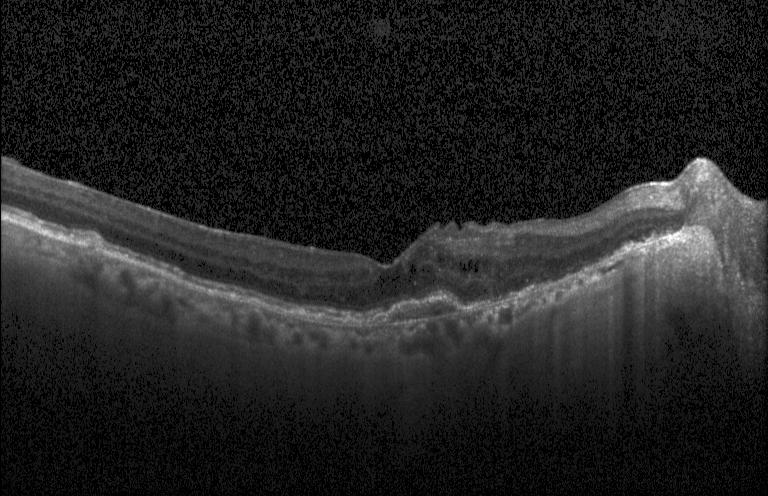

Centered on the fovea; optical coherence tomography scan; spectral-domain optical coherence tomography; Heidelberg Spectralis OCT system — Diagnosis: a choroidal neovascular membrane.